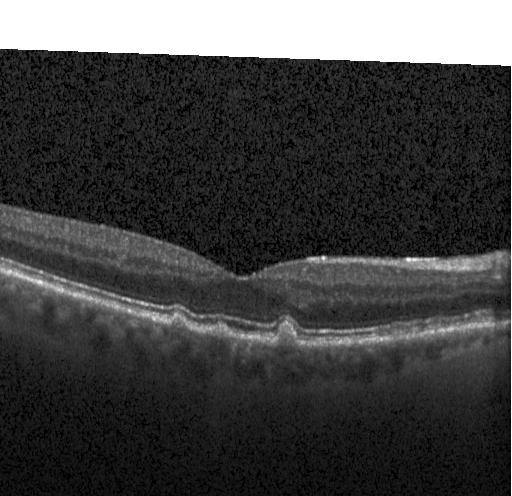

Retinal OCT B-scan
Macular OCT: drusen.